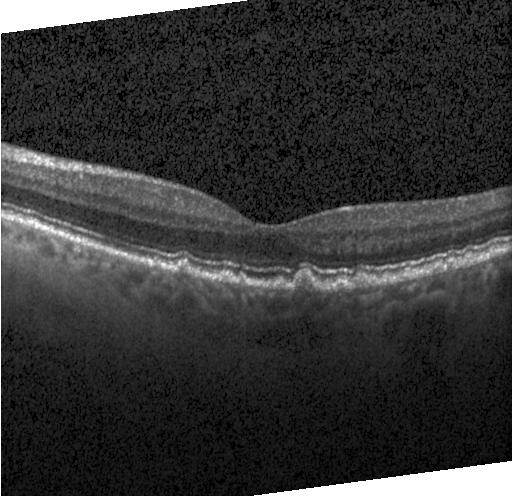

OCT finding: sub-RPE drusenoid deposits.